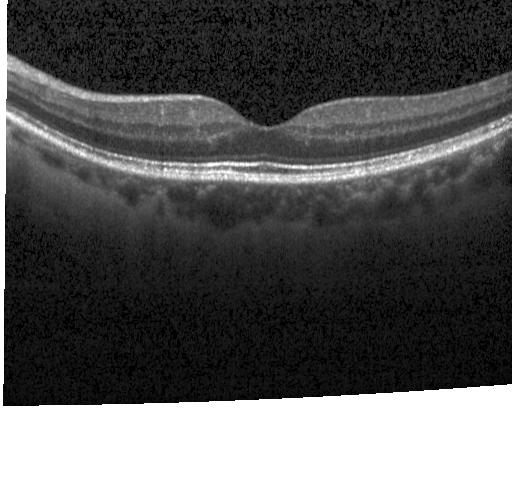
Finding: neither CNV, DME, nor drusen.